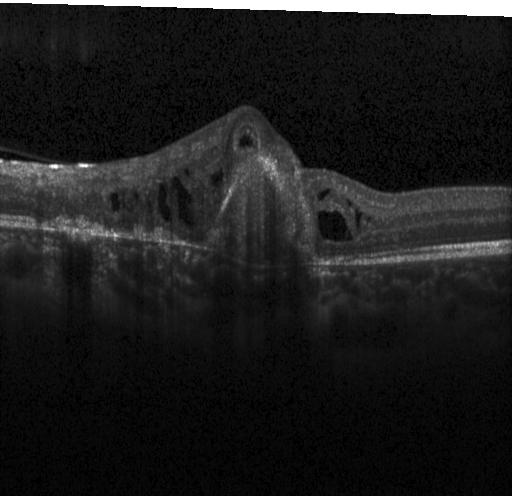

Macular scan · SD-OCT · OCT line scan
A choroidal neovascular membrane.